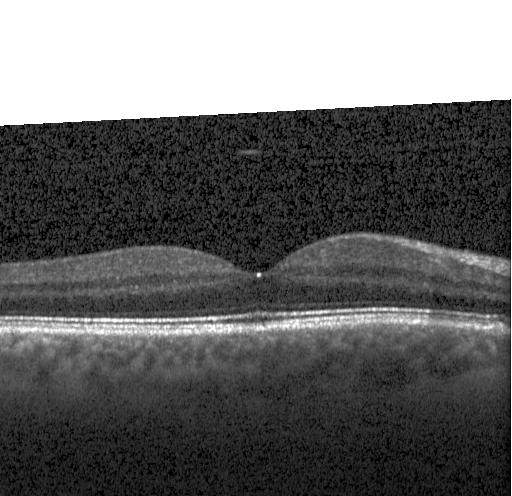
Through the macula, retinal OCT B-scan, Heidelberg Spectralis OCT system. Finding: no choroidal neovascularization, no diabetic macular edema, and no drusen.